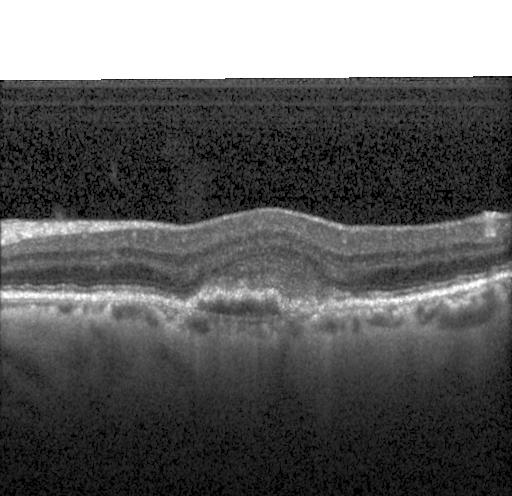
SD-OCT; optical coherence tomography scan. Diagnosis: a choroidal neovascular membrane.